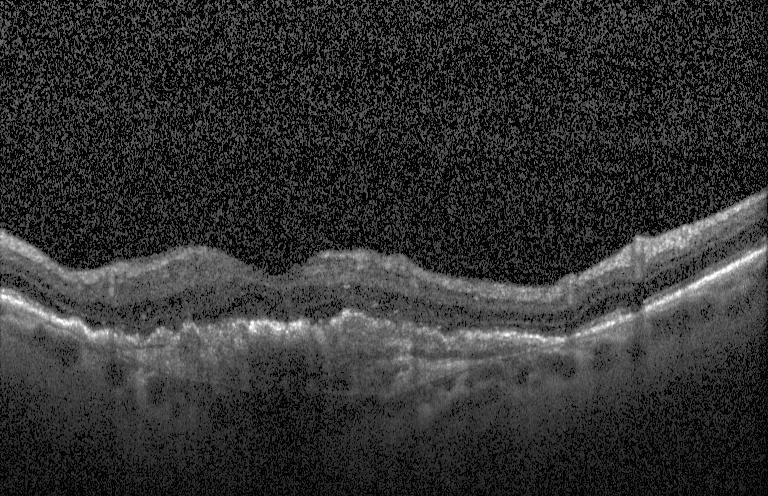

Macular scan · OCT line scan · instrument: Heidelberg Spectralis · SD-OCT.
Diagnosis: choroidal neovascularization (CNV).